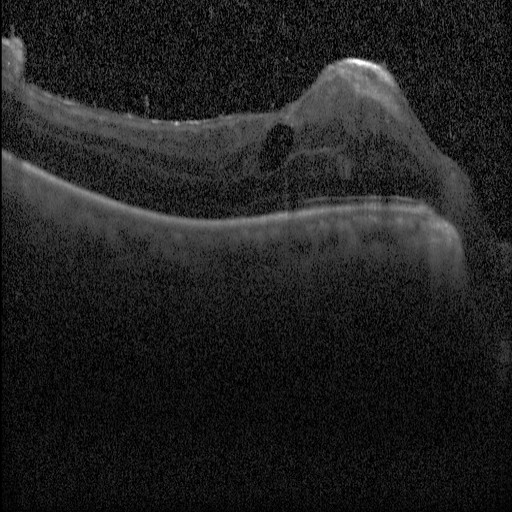

Dx: diabetic macular edema.